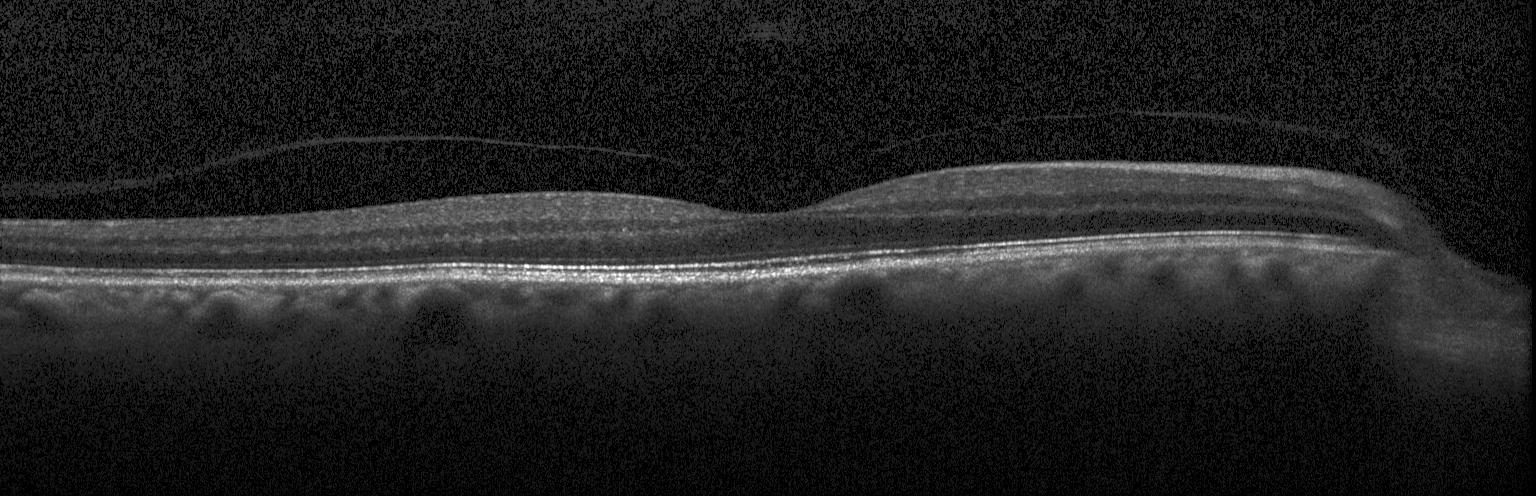

Macular scan · OCT B-scan.
This B-scan demonstrates no choroidal neovascularization, diabetic macular edema, or drusen.